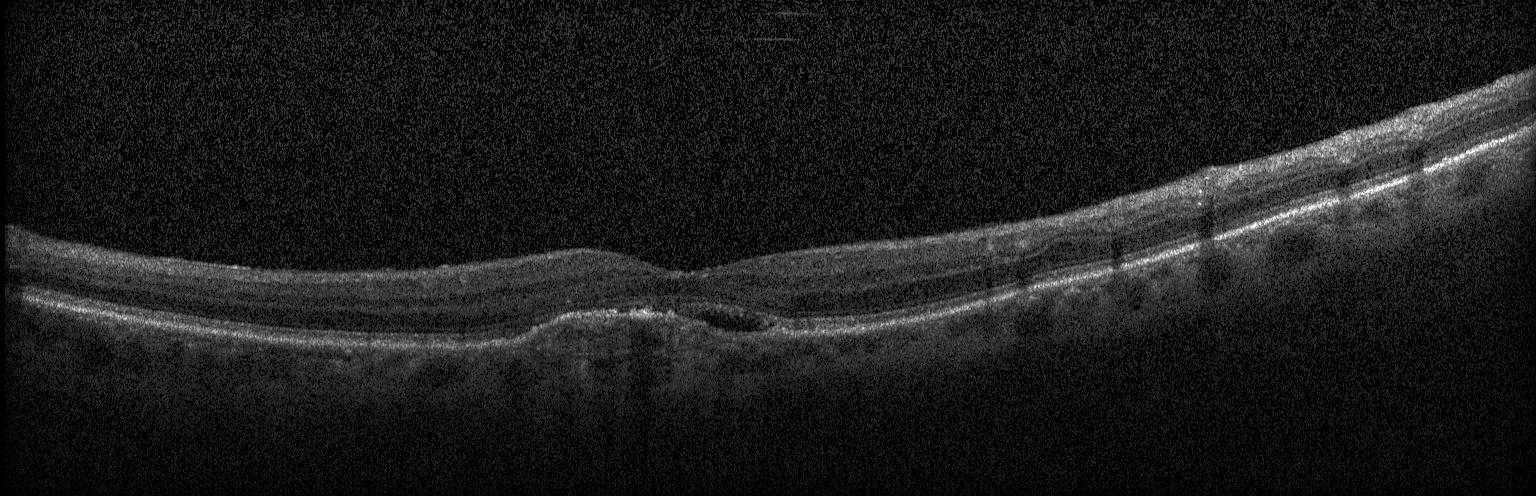
Assessment: a choroidal neovascular membrane.